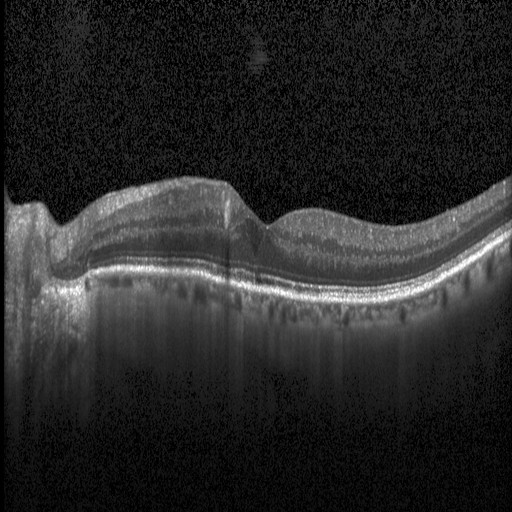 OCT B-scan showing diabetic macular edema (DME).